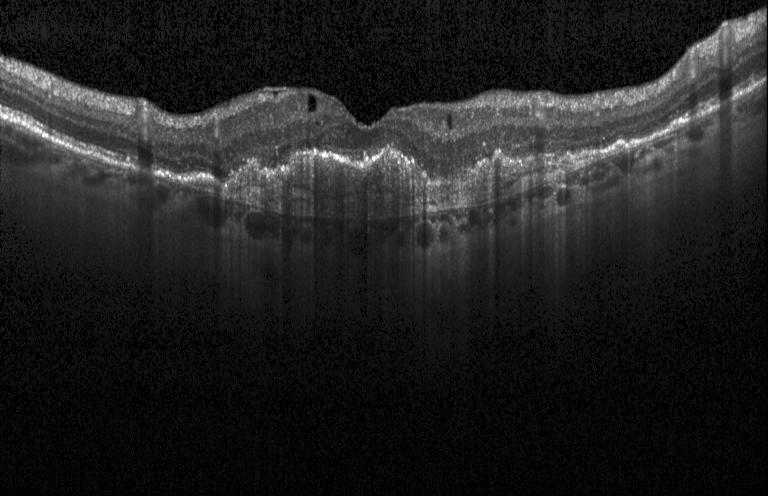
Optical coherence tomography scan; Heidelberg Spectralis
A choroidal neovascular membrane.